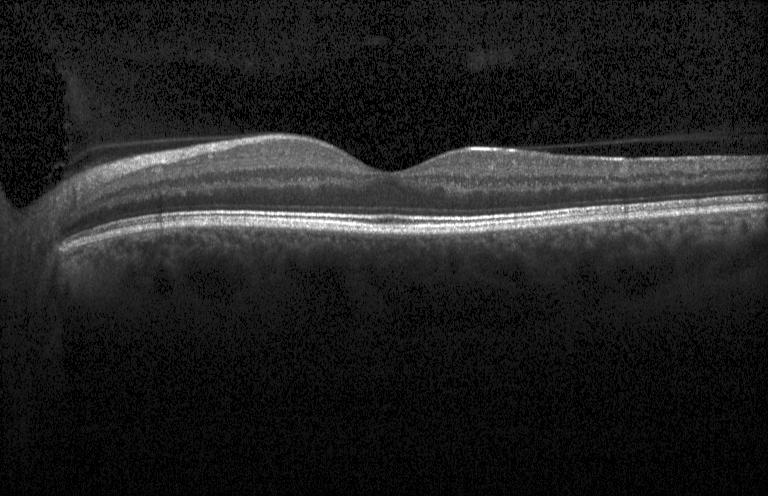

Spectral-domain OCT B-scan: no evidence of choroidal neovascularization, diabetic macular edema, or drusen.